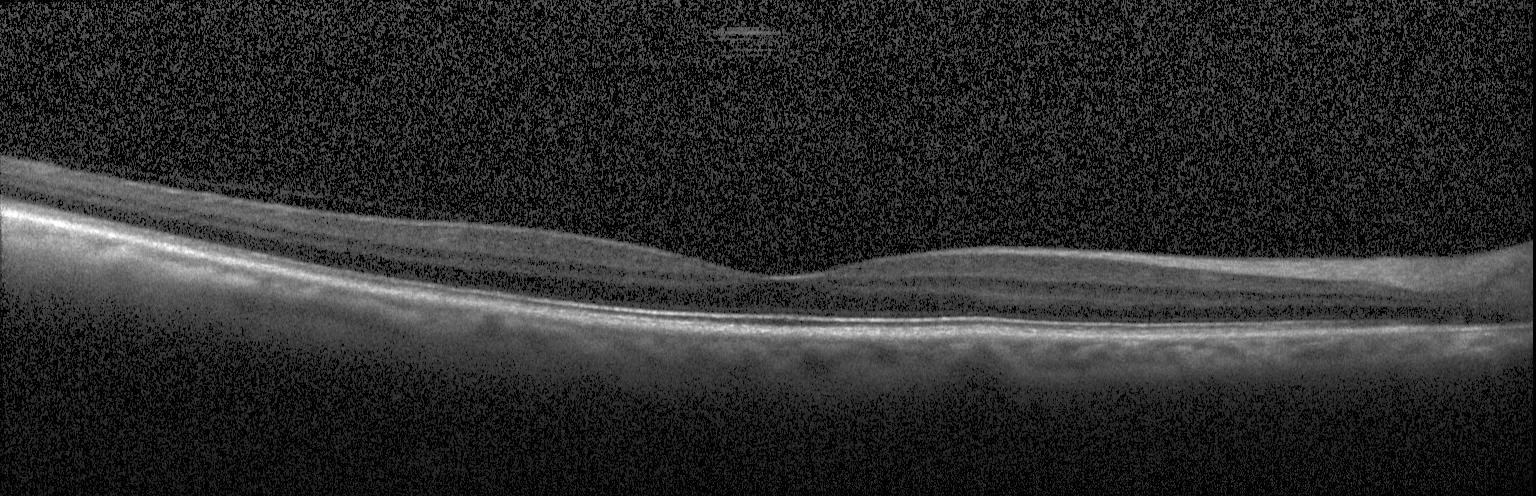
Retinal OCT B-scan. Diagnosis: neither choroidal neovascularization, diabetic macular edema, nor drusen.